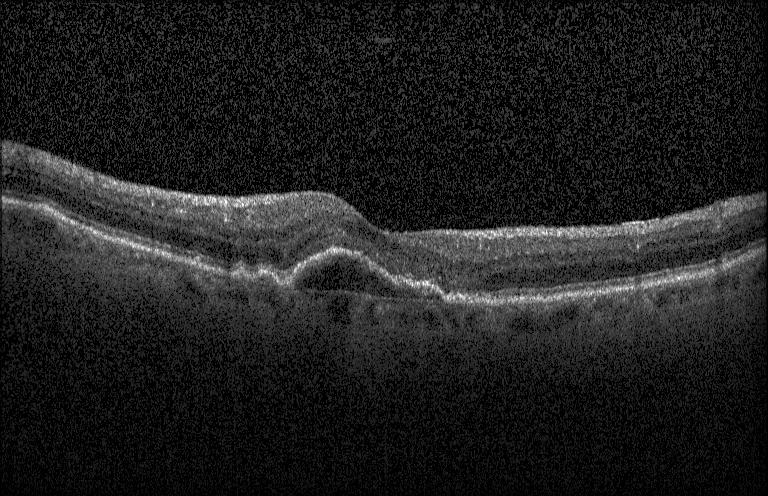

Retinal OCT cross-section · Heidelberg Spectralis OCT system · through the macula
Diagnosis: a choroidal neovascular membrane.